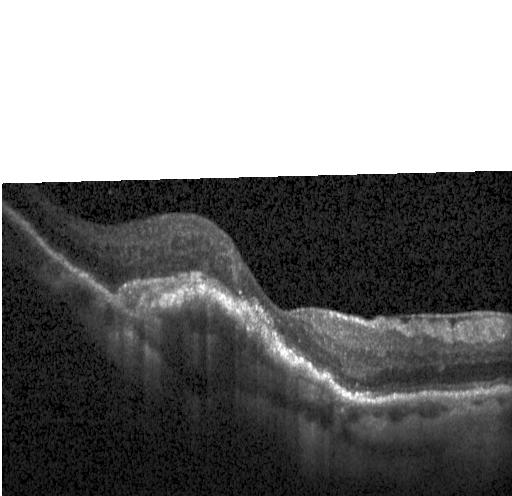
Retinal OCT B-scan. SD-OCT. Through the macula. Heidelberg Spectralis. Assessment: a choroidal neovascular membrane.